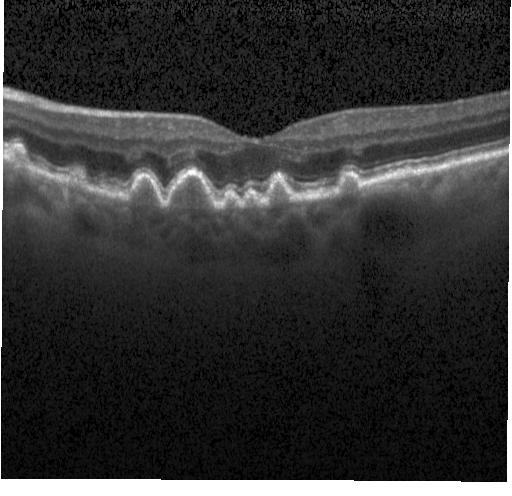
Impression: multiple drusen.